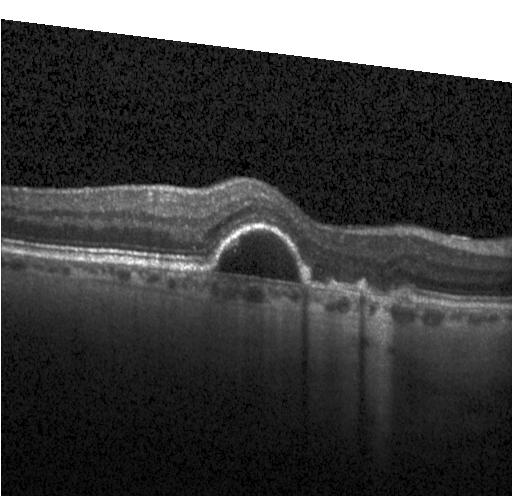
Retinal OCT B-scan.
OCT finding: a choroidal neovascular membrane.